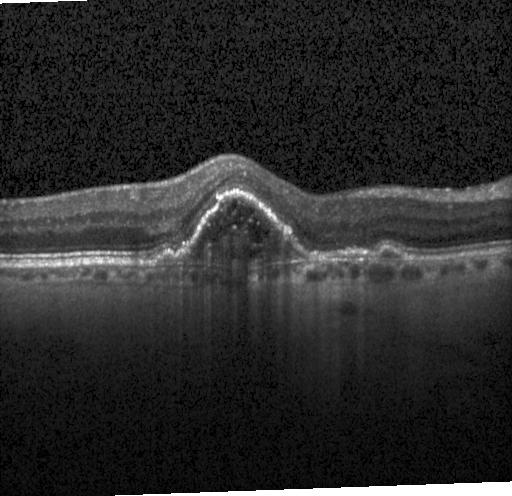 Assessment: a choroidal neovascular membrane.